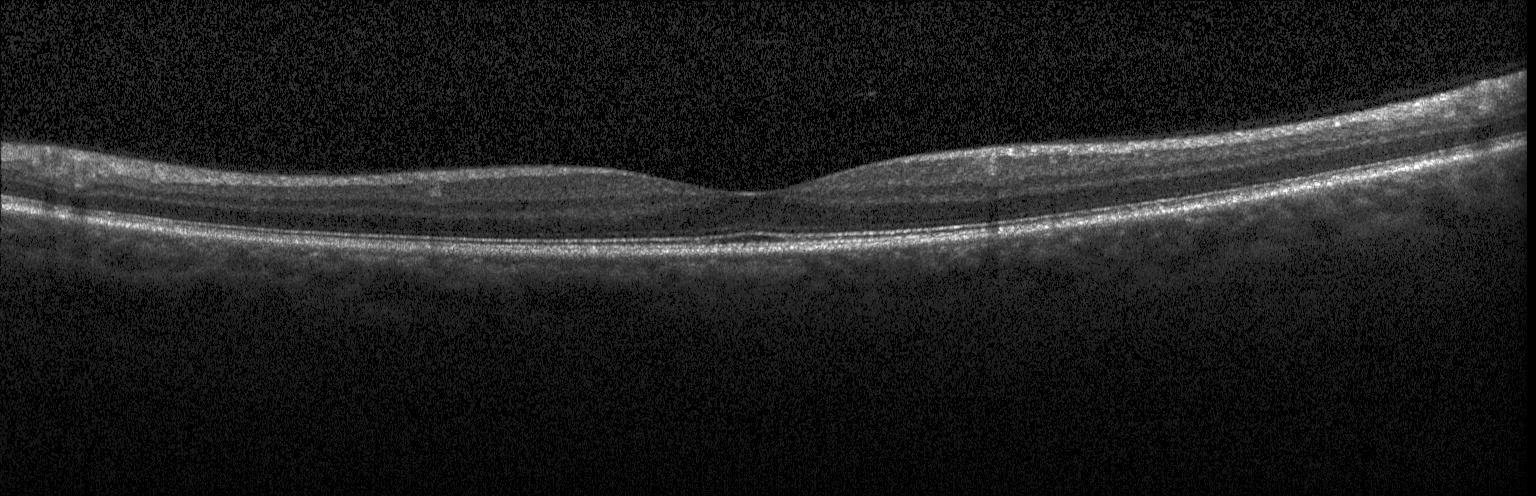

Retinal OCT cross-section
Diagnosis: neither CNV, DME, nor drusen.